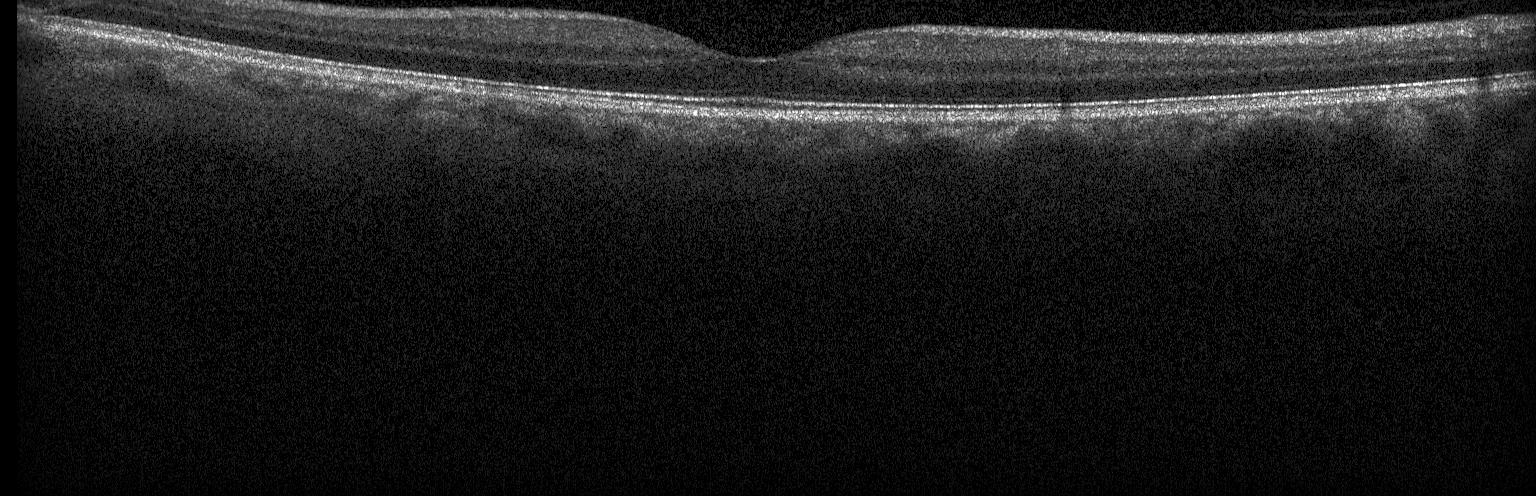 Retinal OCT cross-section · instrument: Heidelberg Spectralis · SD-OCT
OCT finding: neither choroidal neovascularization, diabetic macular edema, nor drusen.